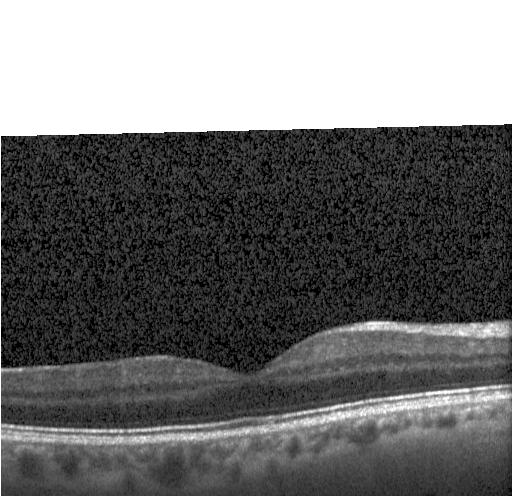

Heidelberg Spectralis OCT system, optical coherence tomography B-scan, fovea-centered, spectral-domain OCT
This B-scan demonstrates no evidence of CNV, DME, or drusen.